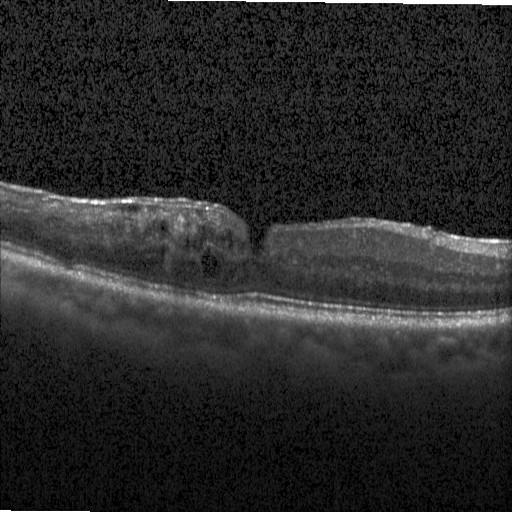

Acquired on a Heidelberg Spectralis · optical coherence tomography scan · horizontal scan through the fovea · spectral-domain optical coherence tomography. Assessment: DME.